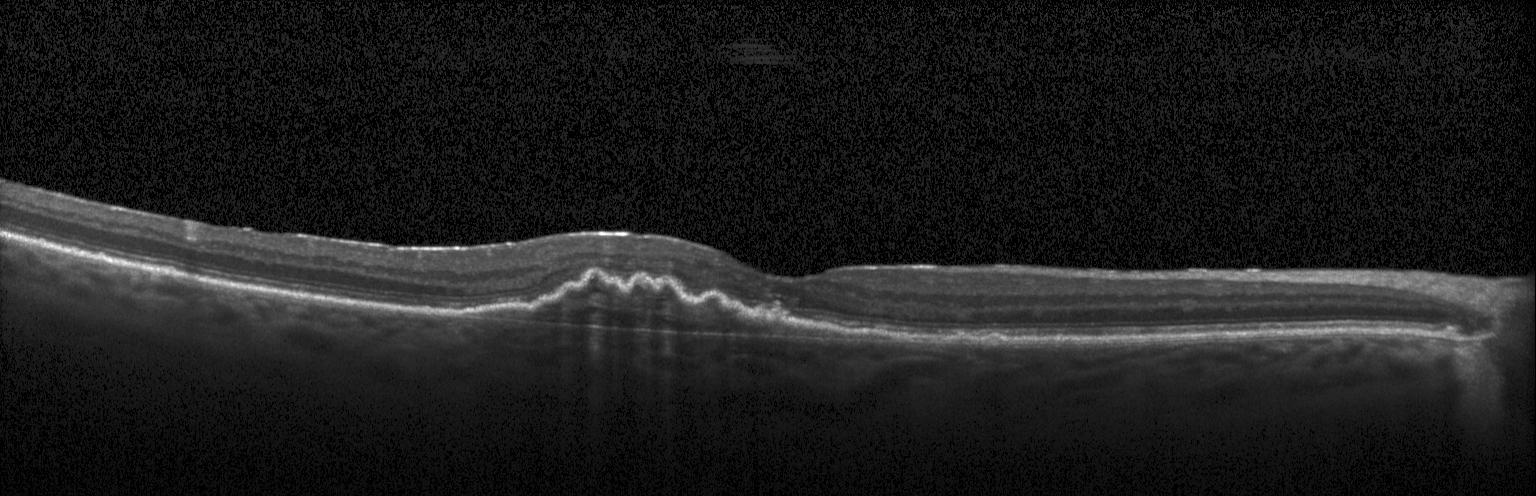 Heidelberg Spectralis OCT system; optical coherence tomography scan
Macular OCT: a choroidal neovascular membrane.